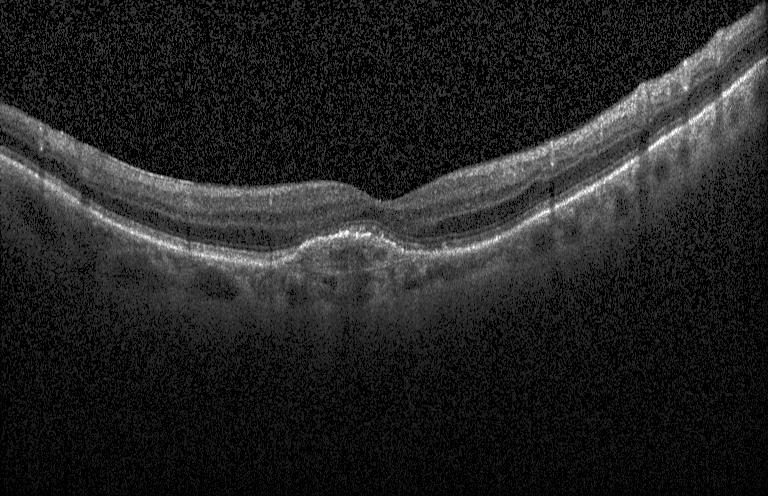
Diagnosis: choroidal neovascularization.